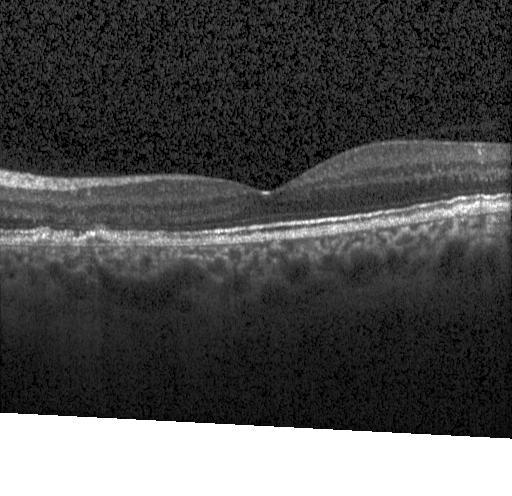
Macular OCT demonstrating a choroidal neovascular membrane.